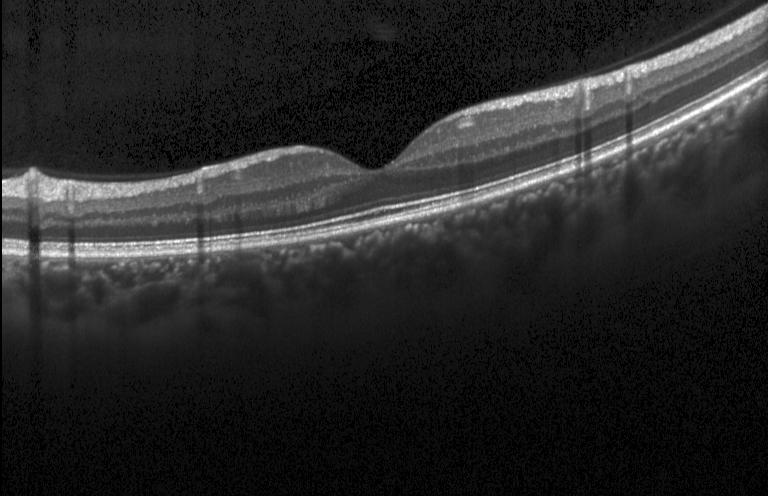
Optical coherence tomography scan — The scan shows no choroidal neovascularization, diabetic macular edema, or drusen.